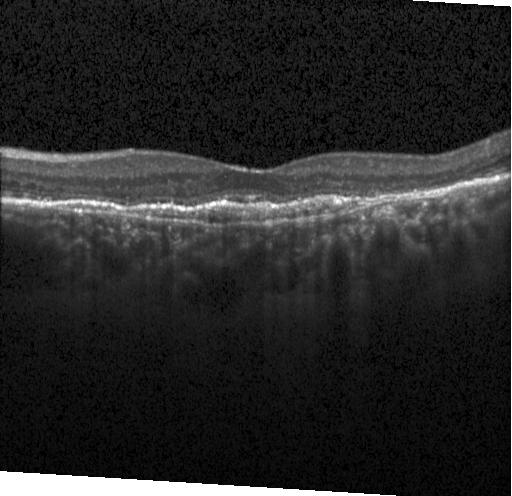 A choroidal neovascular membrane.